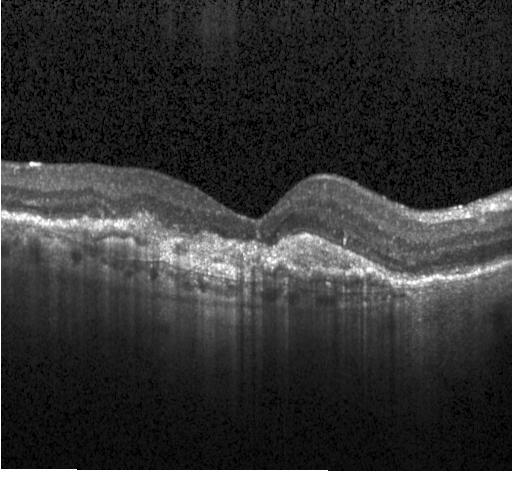 Spectral-domain OCT. Instrument: Heidelberg Spectralis. Macular scan. Retinal OCT cross-section — Finding: a choroidal neovascular membrane.